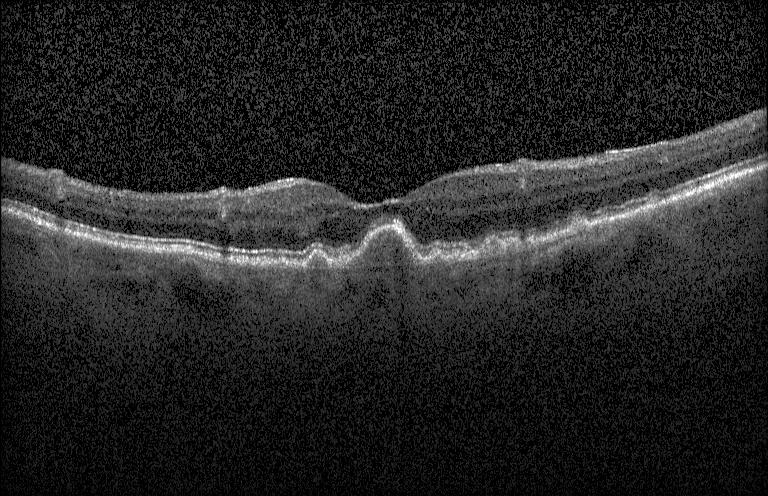 This B-scan demonstrates multiple drusen.